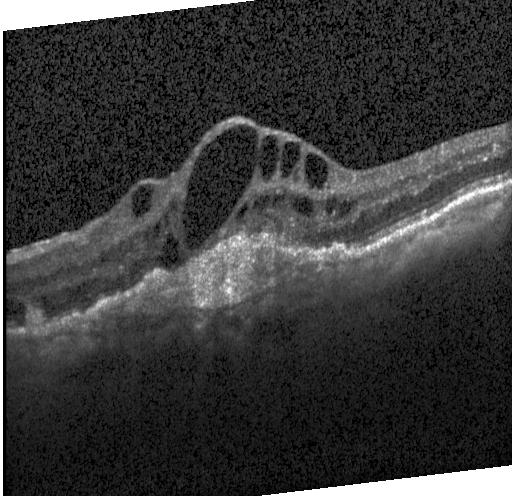
Acquired on a Heidelberg Spectralis. Fovea-centered. Optical coherence tomography B-scan — Macular OCT: a choroidal neovascular membrane.